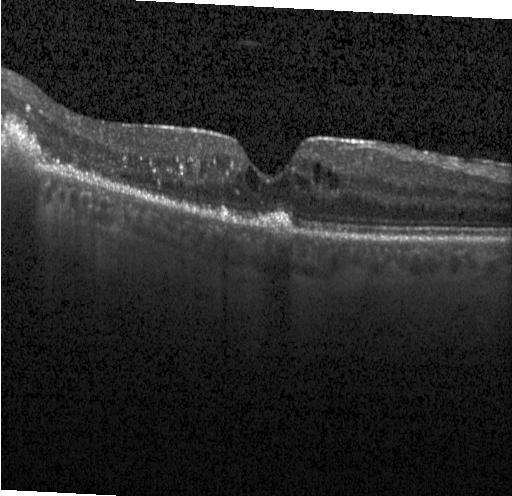

Retinal OCT cross-section
Choroidal neovascularization.